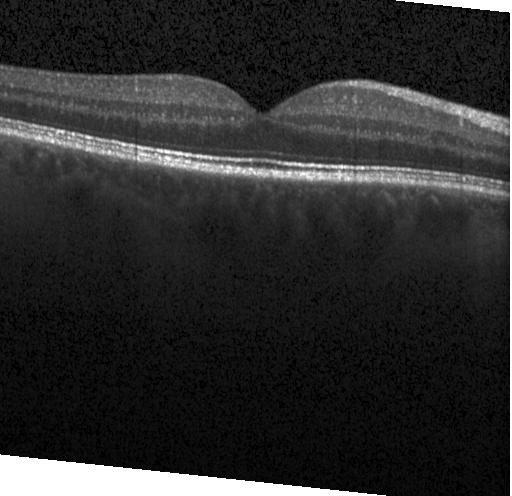 OCT finding: no evidence of choroidal neovascularization, diabetic macular edema, or drusen.